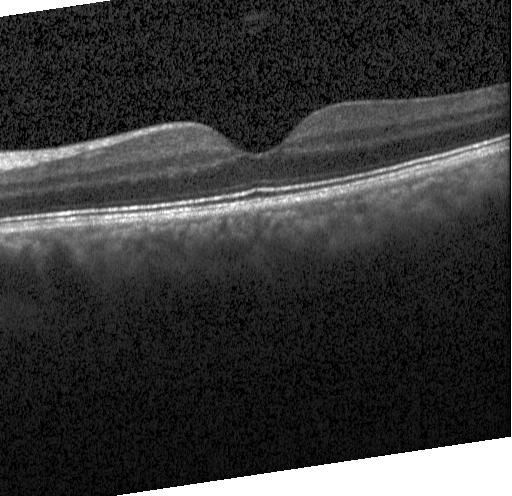

Through the macula; optical coherence tomography scan; instrument: Heidelberg Spectralis. Impression: no choroidal neovascularization, no diabetic macular edema, and no drusen.